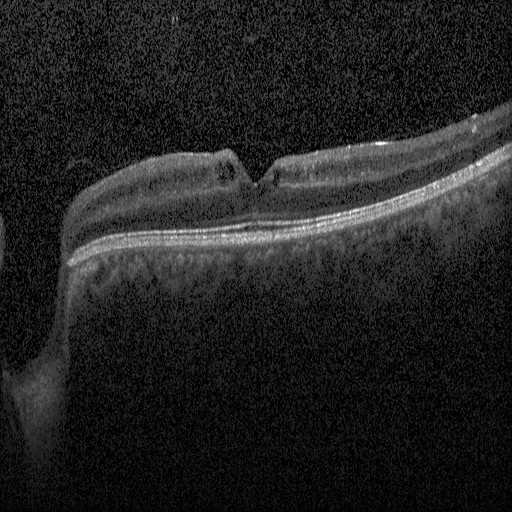
OCT line scan — Impression: diabetic macular edema.